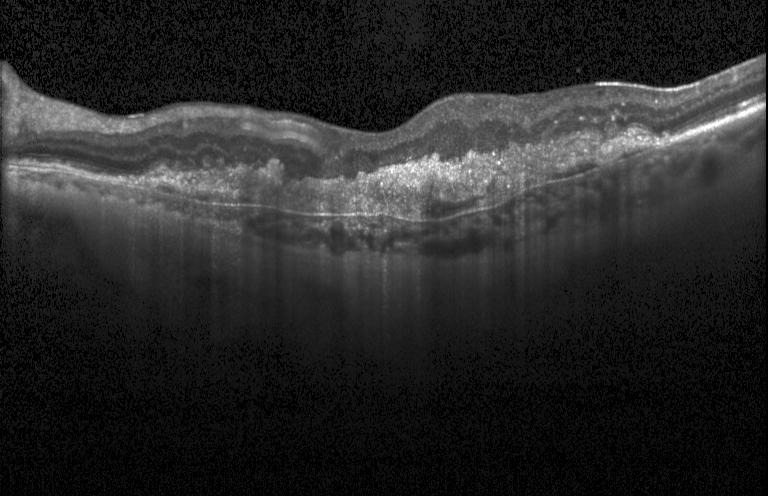 OCT line scan. Through the macula — Diagnosis: a choroidal neovascular membrane.